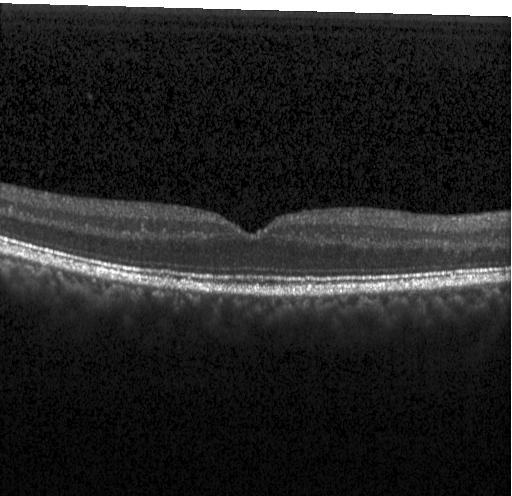 Acquired on a Heidelberg Spectralis. Macular scan. OCT line scan — Diagnosis: no CNV, no DME, and no drusen.